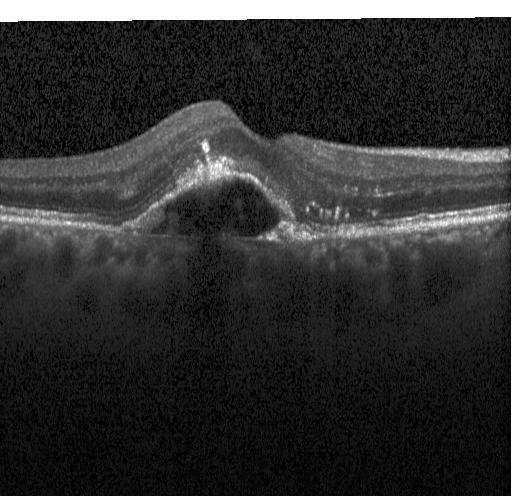 Retinal OCT B-scan.
Finding: a choroidal neovascular membrane.